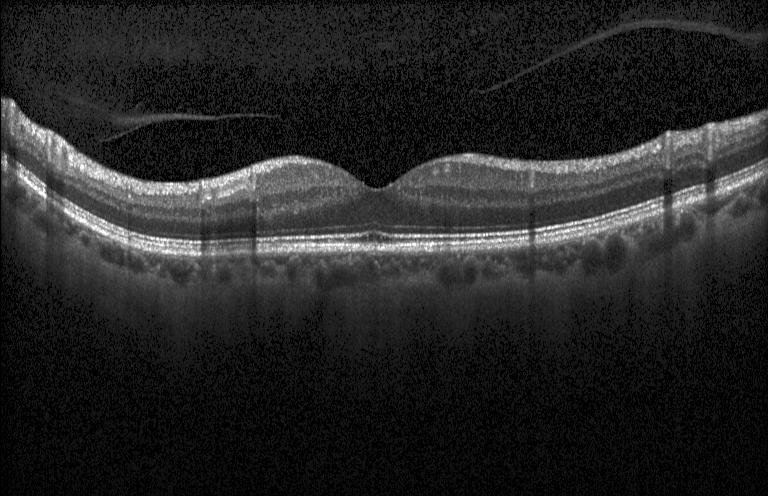

Assessment: no evidence of choroidal neovascularization, diabetic macular edema, or drusen.